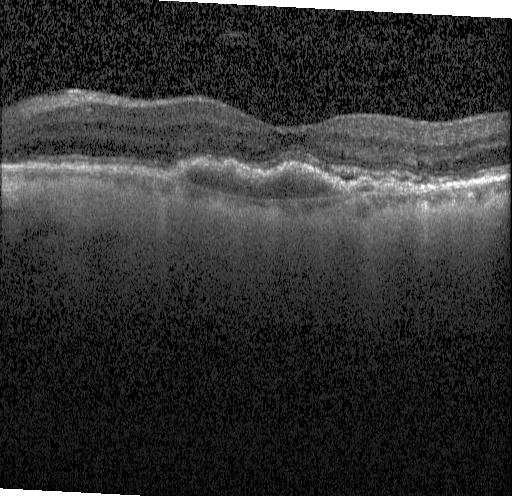
Spectral-domain optical coherence tomography; Heidelberg Spectralis OCT system; optical coherence tomography B-scan — Assessment: a choroidal neovascular membrane.